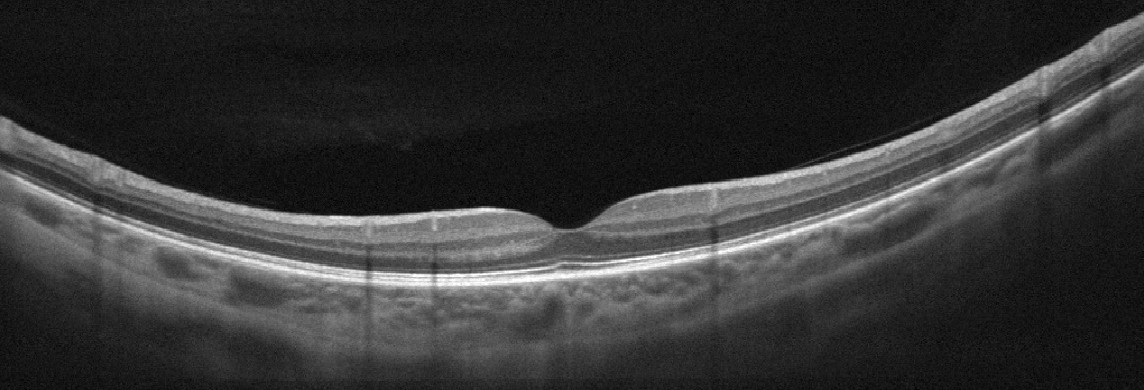 Acquired on an Optovue Avanti RTVue XR. Macular scan. OCT line scan
Absence of AMD, DME, ERM, RAO, RVO, and vitreomacular interface disease.